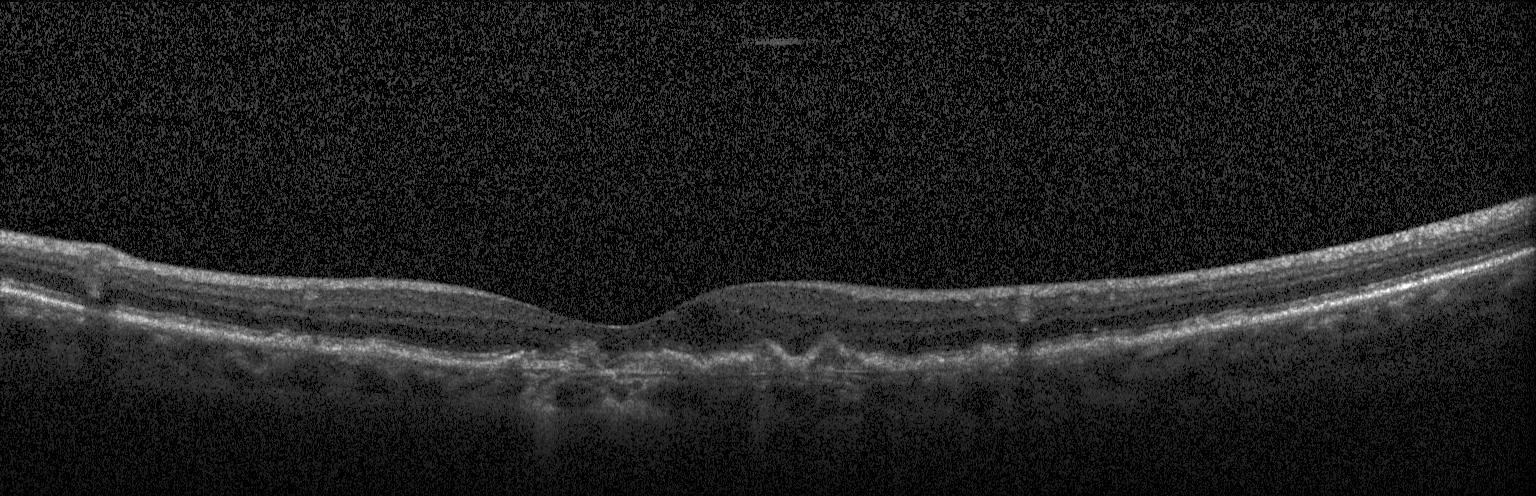 This B-scan demonstrates a choroidal neovascular membrane.